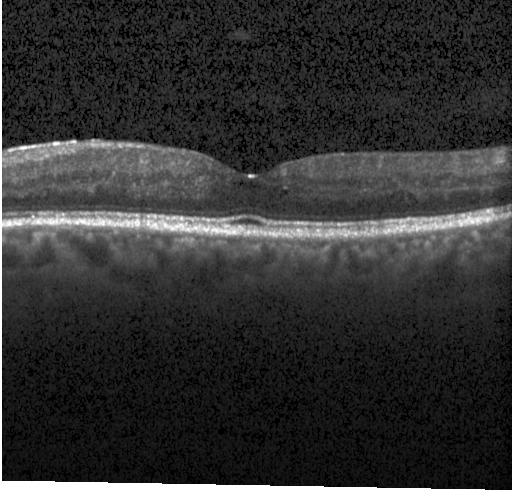
Finding: no choroidal neovascularization, diabetic macular edema, or drusen.